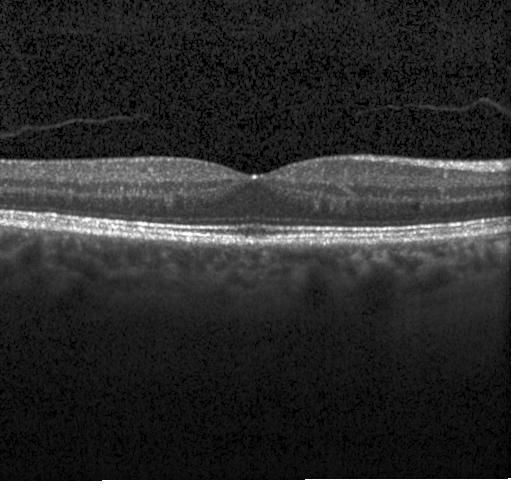 OCT finding: no choroidal neovascularization, no diabetic macular edema, and no drusen.